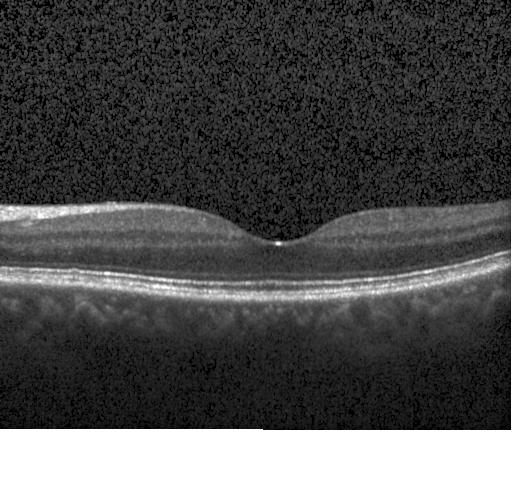 Retinal OCT B-scan. Centered on the fovea. Spectral-domain optical coherence tomography
Finding: neither CNV, DME, nor drusen.